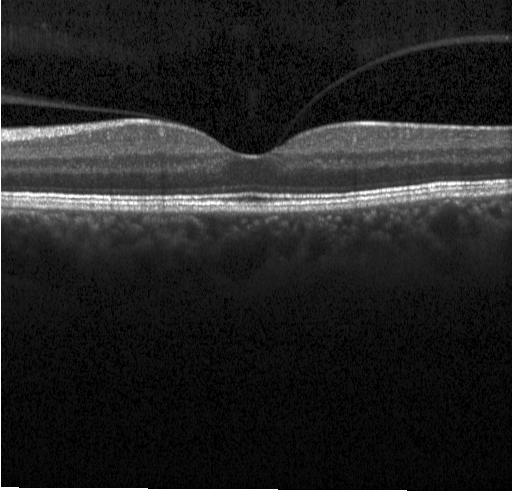

Spectral-domain OCT · OCT line scan · macular scan · acquired on a Heidelberg Spectralis. Diagnosis: neither choroidal neovascularization, diabetic macular edema, nor drusen.